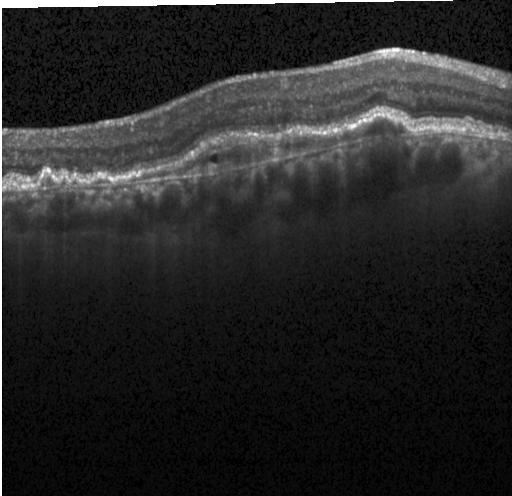

Through the macula, SD-OCT, OCT line scan. Diagnosis: a choroidal neovascular membrane.